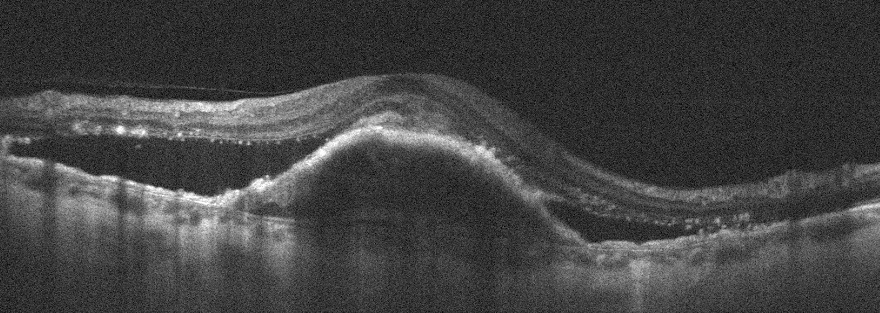
This B-scan demonstrates AMD.